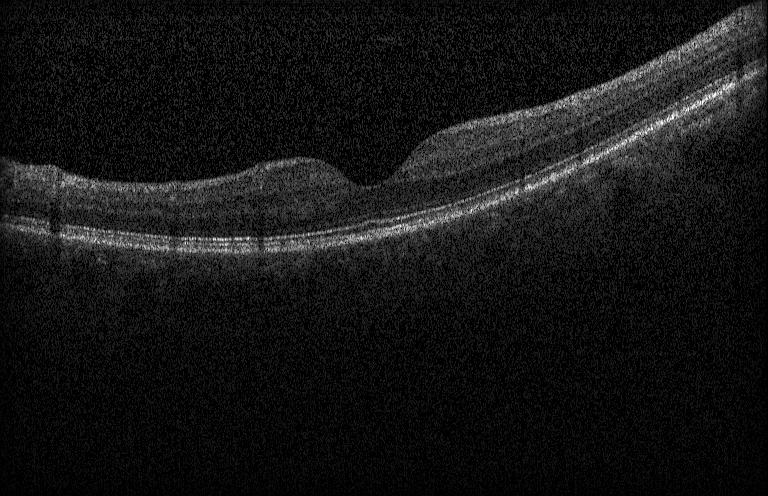
Instrument: Heidelberg Spectralis. Optical coherence tomography scan. Spectral-domain OCT. Macular scan.
Dx: no evidence of choroidal neovascularization, diabetic macular edema, or drusen.